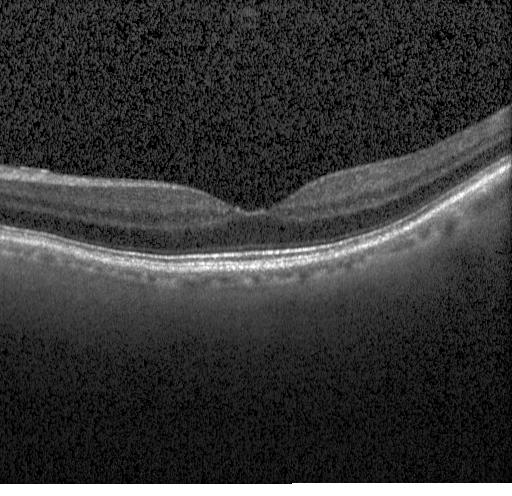

Retinal OCT cross-section. Heidelberg Spectralis OCT system. SD-OCT — Diagnosis: no choroidal neovascularization, no diabetic macular edema, and no drusen.